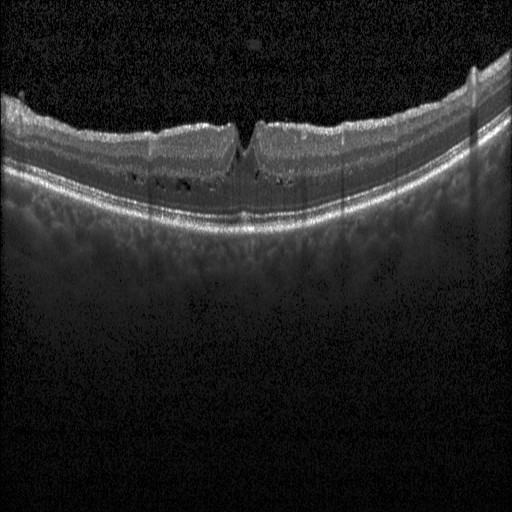
Retinal OCT cross-section — Finding: diabetic macular edema.